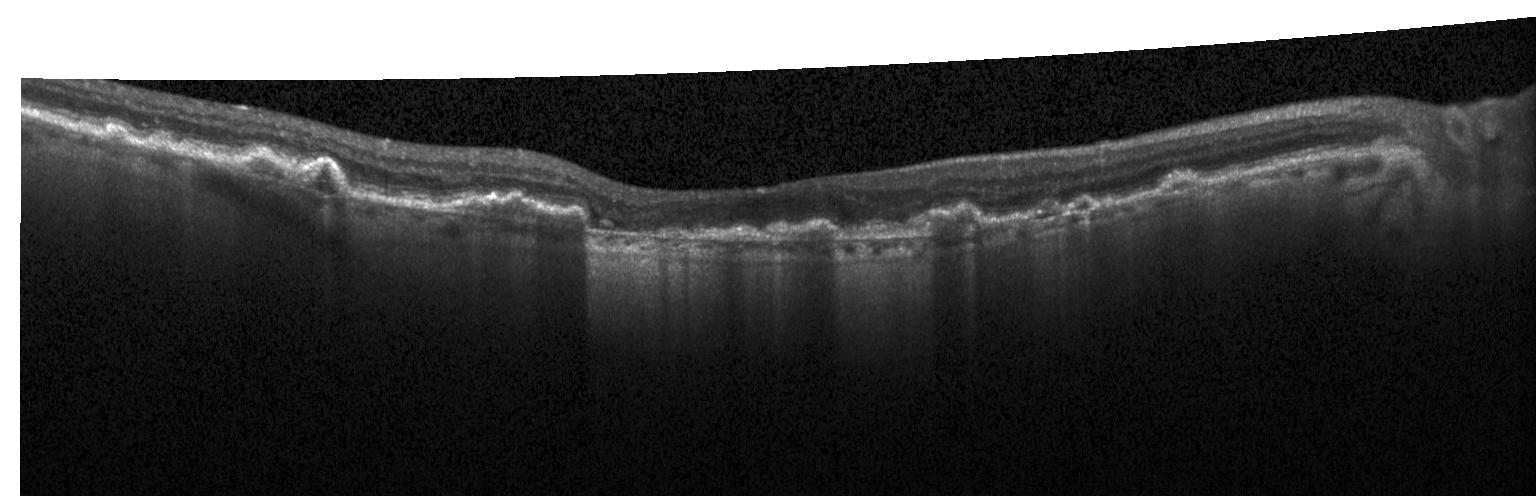
This B-scan demonstrates a choroidal neovascular membrane.